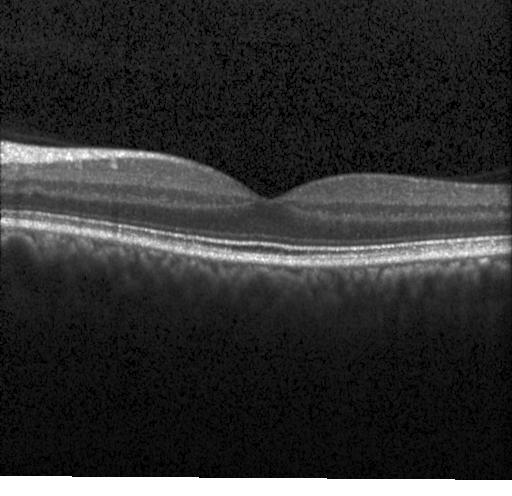 Retinal OCT cross-section.
Macular OCT: neither choroidal neovascularization, diabetic macular edema, nor drusen.